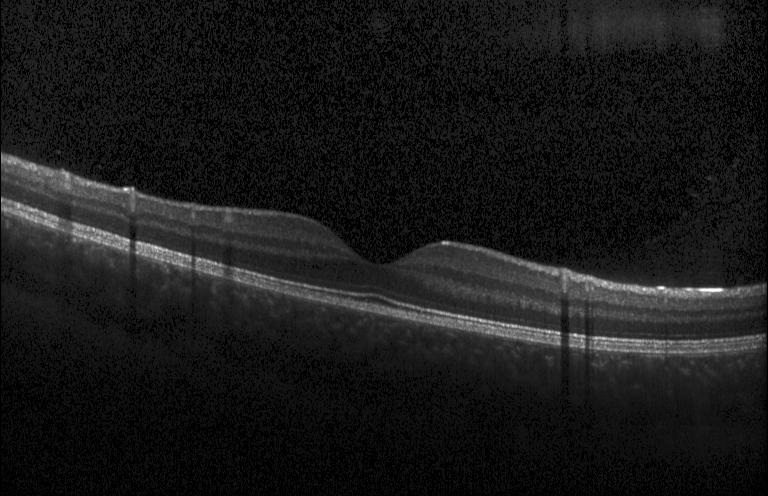
The scan shows no evidence of CNV, DME, or drusen.